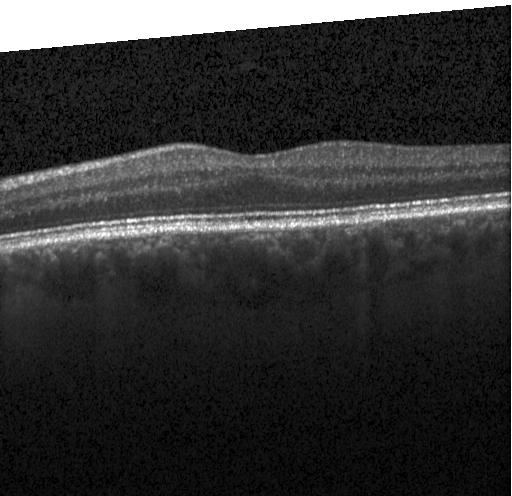

Diagnosis: no CNV, DME, or drusen.